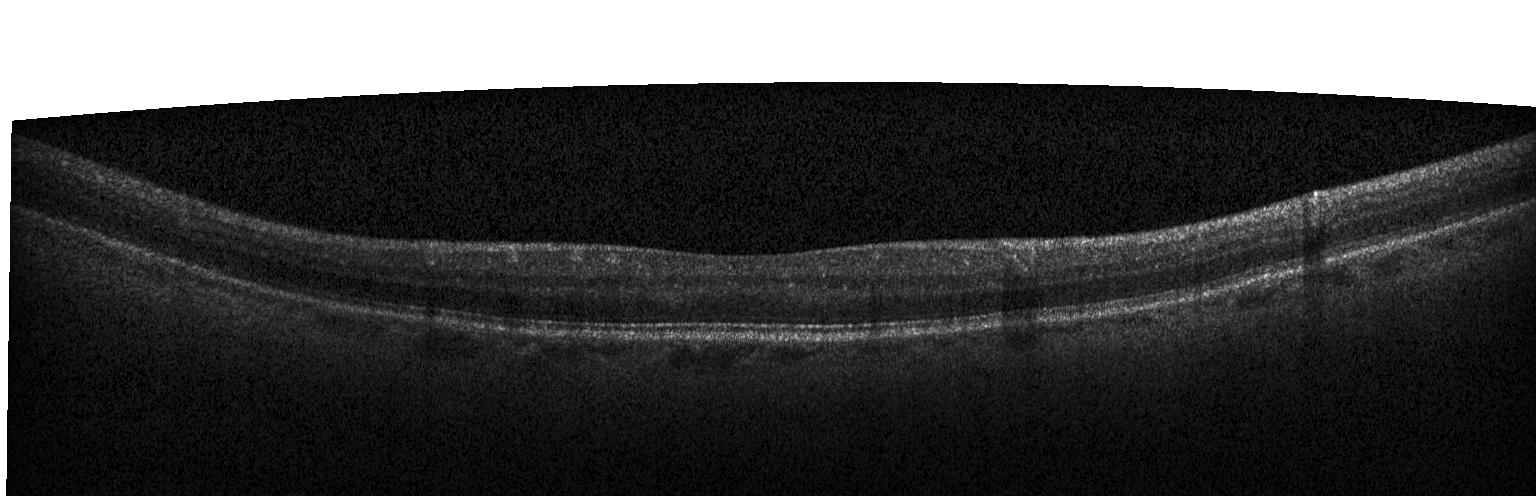 Impression: neither choroidal neovascularization, diabetic macular edema, nor drusen.